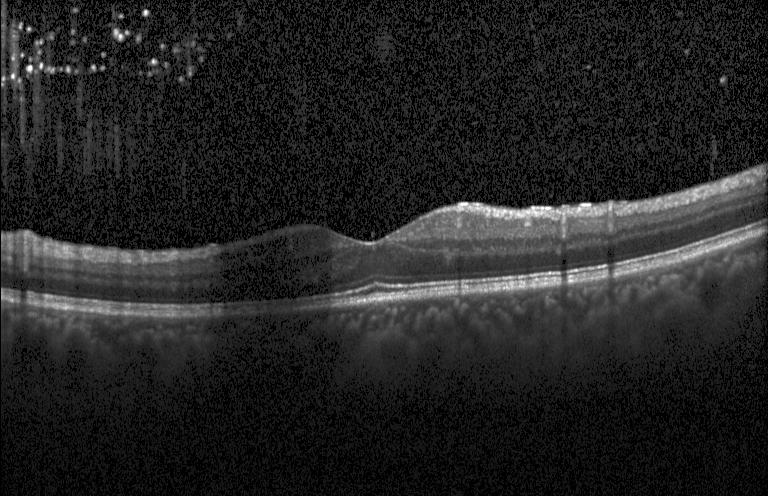
Through the macula. OCT B-scan — Assessment: no choroidal neovascularization, no diabetic macular edema, and no drusen.